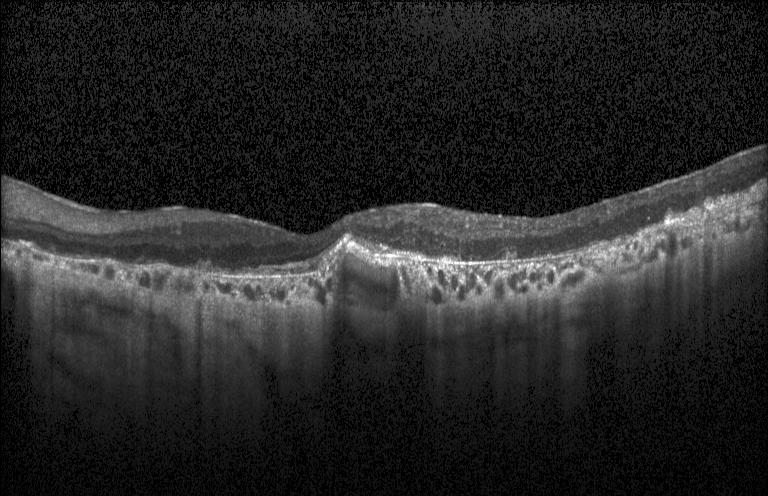
Optical coherence tomography B-scan. Horizontal scan through the fovea. Instrument: Heidelberg Spectralis
Diagnosis: a choroidal neovascular membrane.